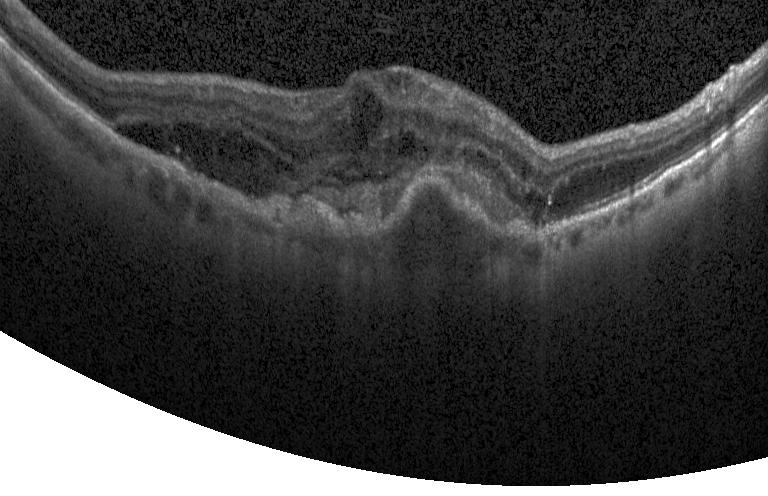

Optical coherence tomography scan
Finding: a choroidal neovascular membrane.